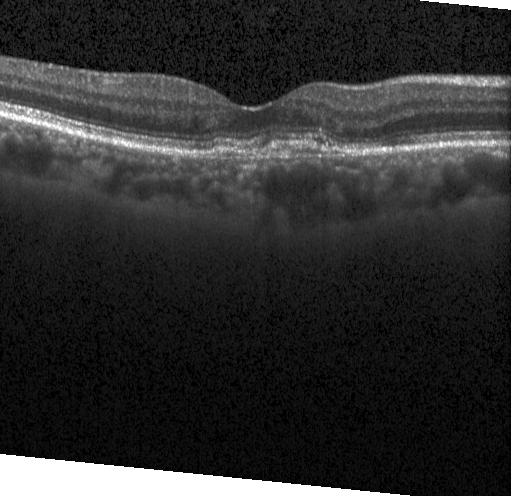 Retinal OCT cross-section. Dx: a choroidal neovascular membrane.